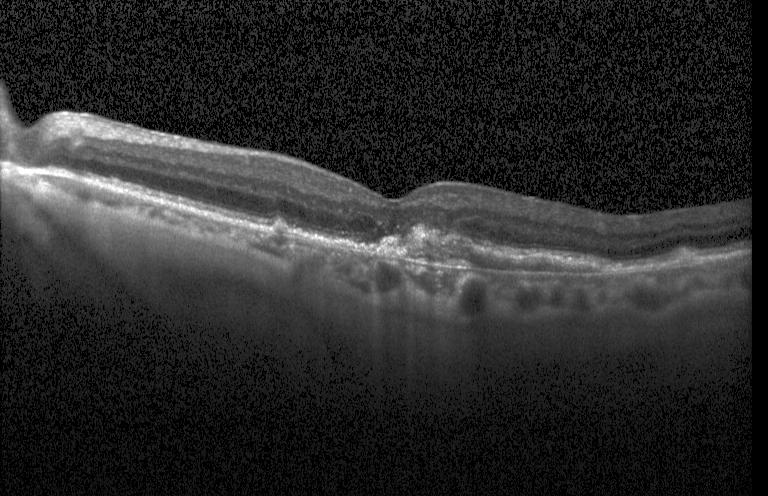
OCT B-scan — A choroidal neovascular membrane.